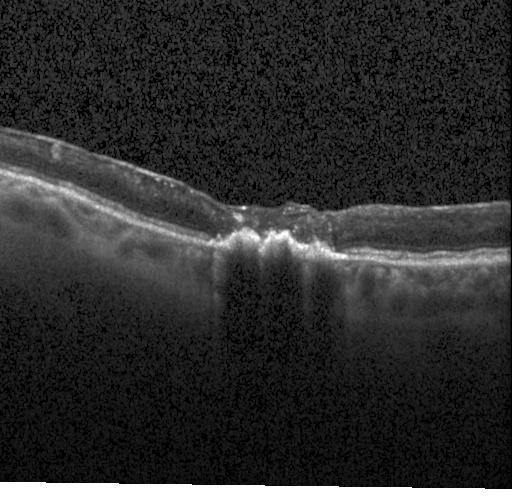
Spectral-domain OCT B-scan: a choroidal neovascular membrane.